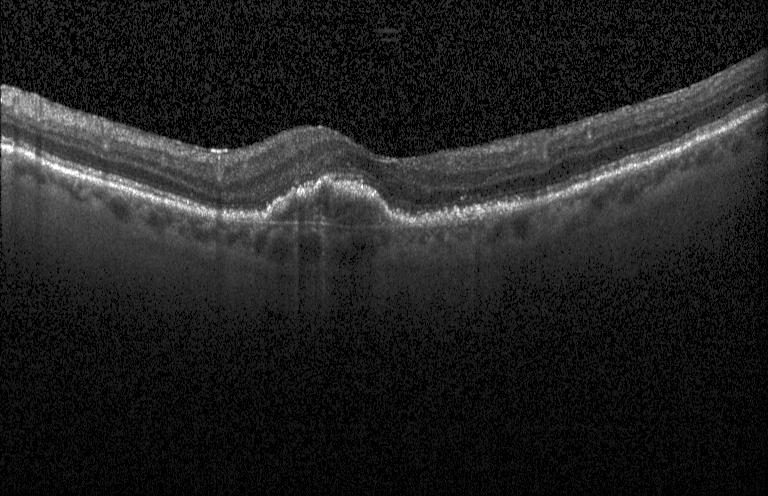 Optical coherence tomography scan — Diagnosis: a choroidal neovascular membrane.